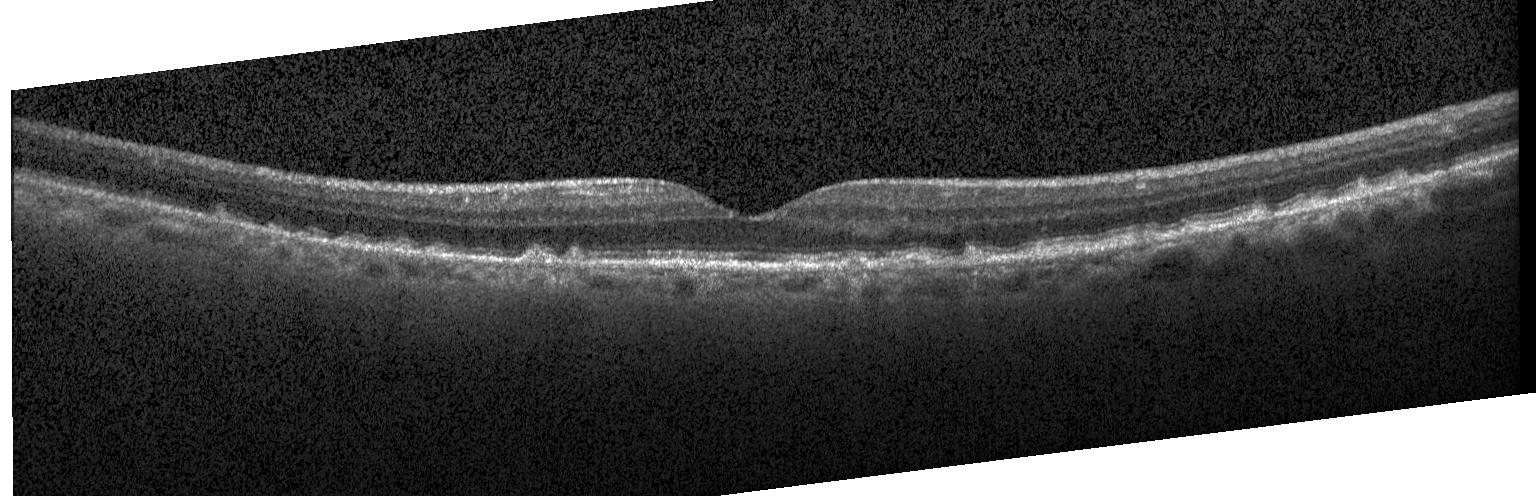

Spectral-domain OCT. OCT B-scan. Finding: multiple drusen.